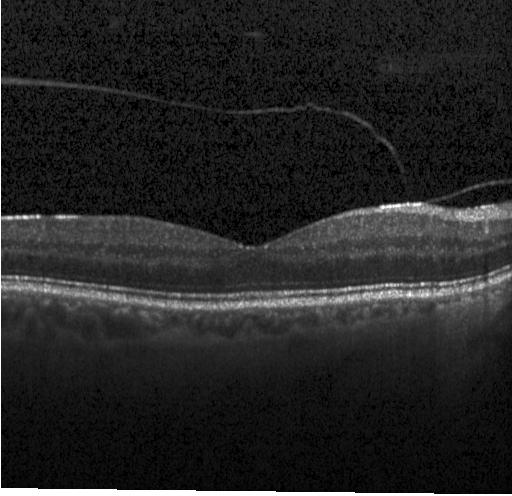 OCT B-scan · centered on the fovea. No CNV, DME, or drusen.